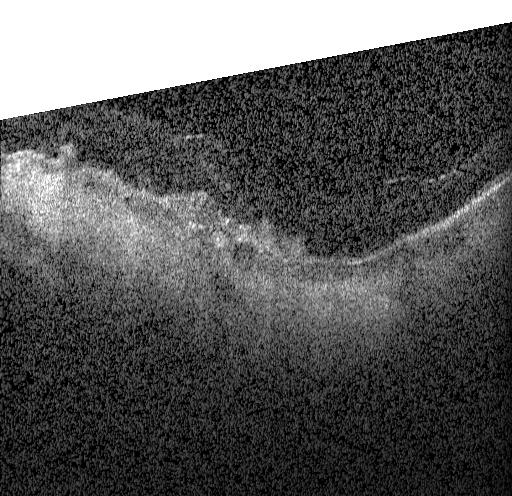 Acquired on a Heidelberg Spectralis · spectral-domain optical coherence tomography · OCT B-scan. Diagnosis: a choroidal neovascular membrane.